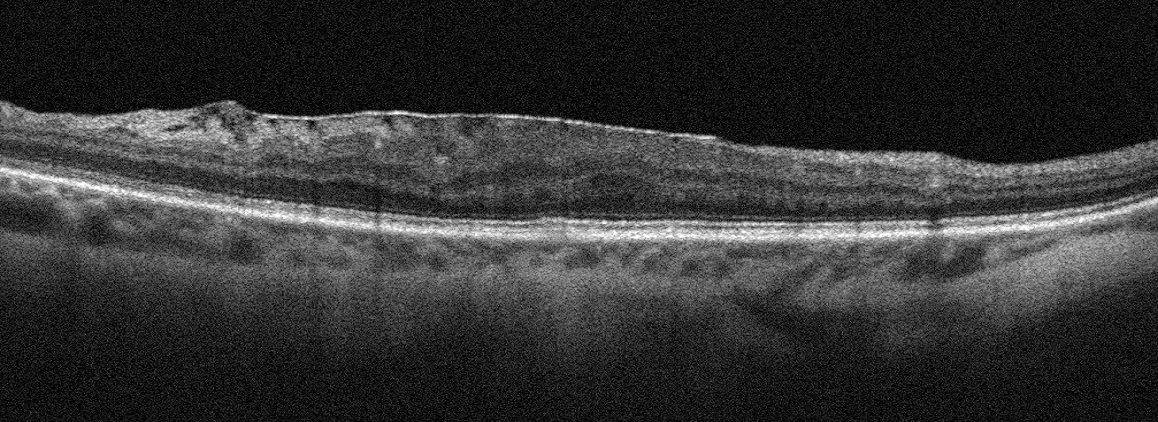
Through the macula, OCT line scan, acquired on an Optovue Avanti RTVue XR, oculus sinister.
Macular OCT: epiretinal membrane (ERM).